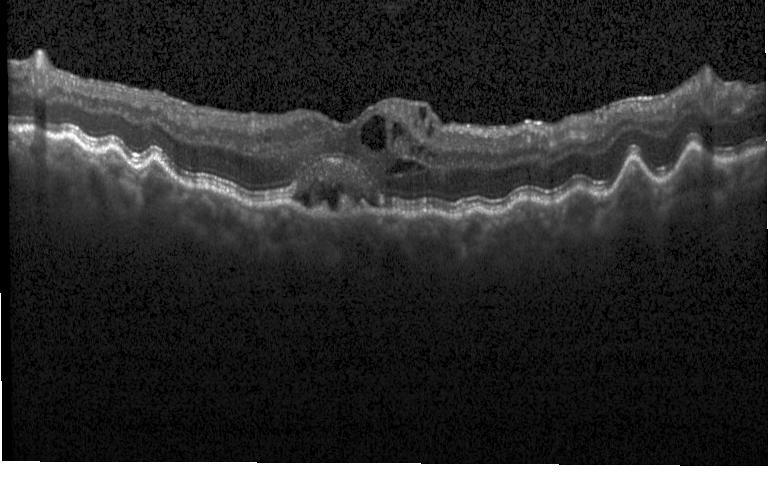
Macular OCT demonstrating CNV.